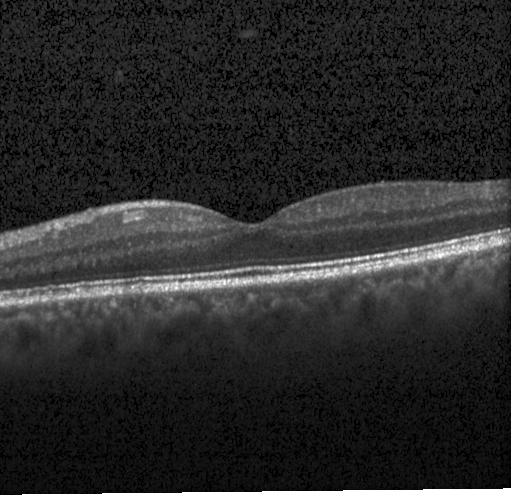 Spectral-domain OCT B-scan: no choroidal neovascularization, no diabetic macular edema, and no drusen.